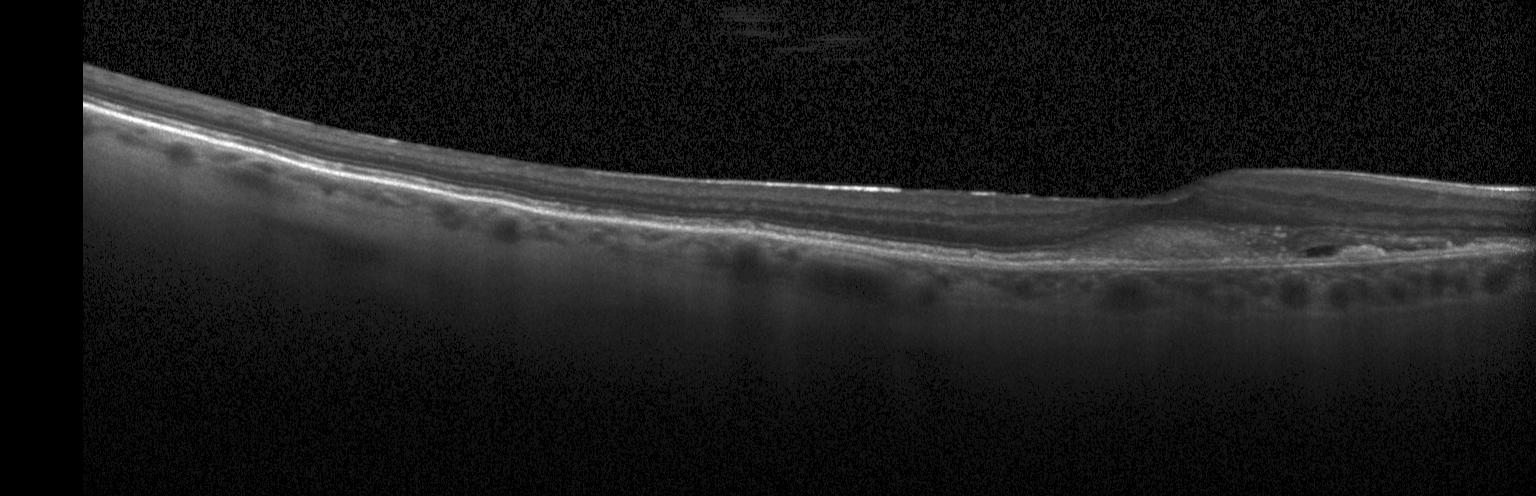 Optical coherence tomography B-scan · Heidelberg Spectralis OCT system · SD-OCT.
OCT finding: choroidal neovascularization.